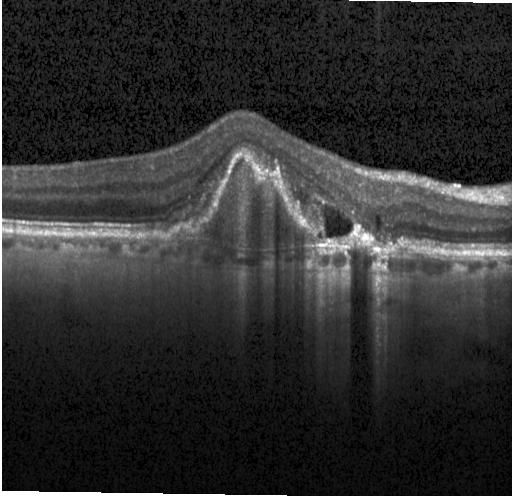
Assessment: choroidal neovascularization.